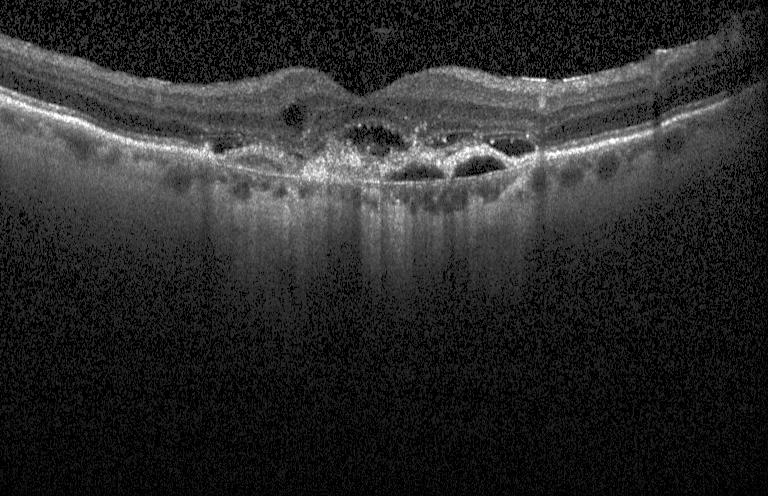
Centered on the fovea. Optical coherence tomography scan
CNV.